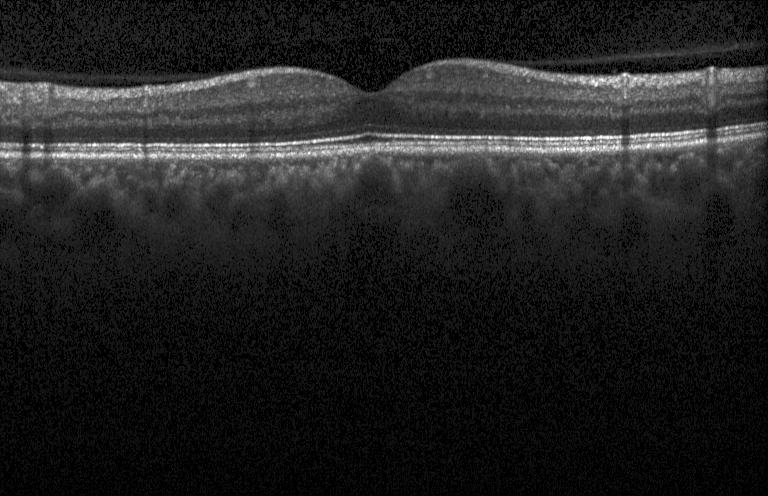

Dx: no evidence of CNV, DME, or drusen.